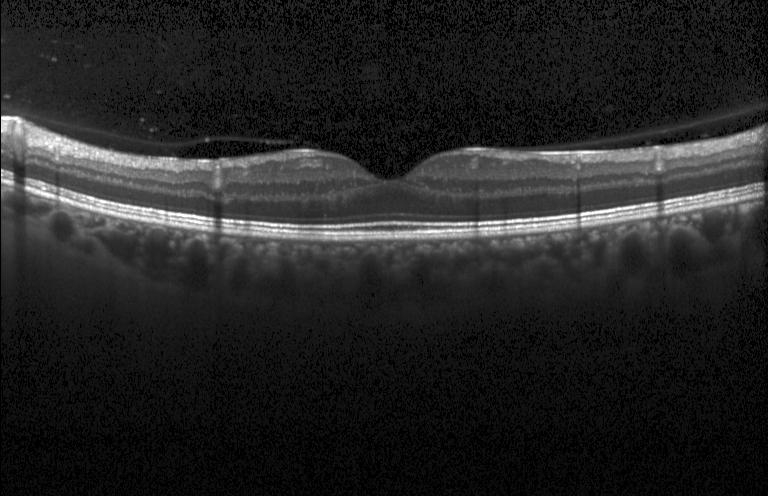 Retinal OCT B-scan
Macular OCT: no evidence of choroidal neovascularization, diabetic macular edema, or drusen.